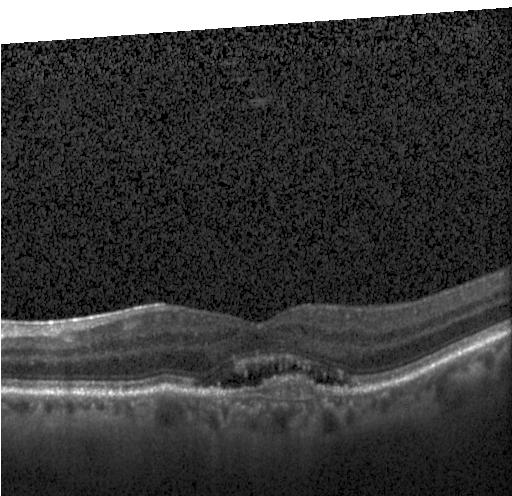

OCT B-scan · Heidelberg Spectralis OCT system · centered on the fovea · spectral-domain OCT. Impression: choroidal neovascularization.